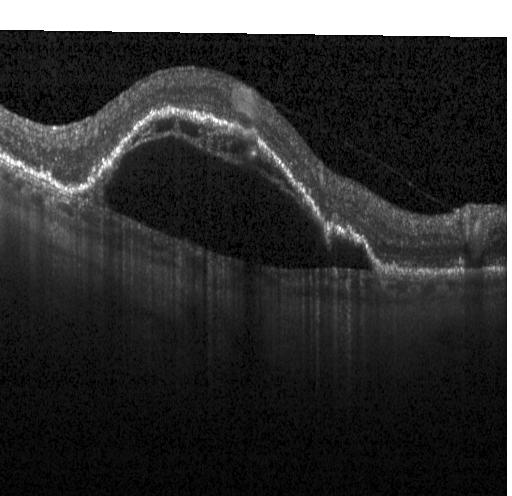 Finding: choroidal neovascularization.